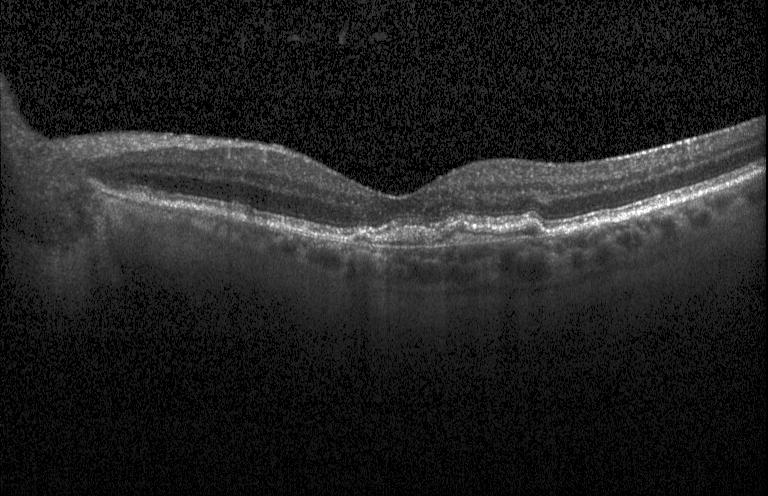
Retinal OCT cross-section showing CNV.